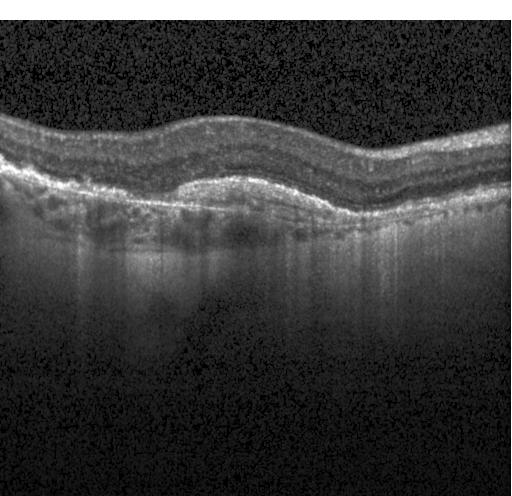 OCT scan showing a choroidal neovascular membrane.